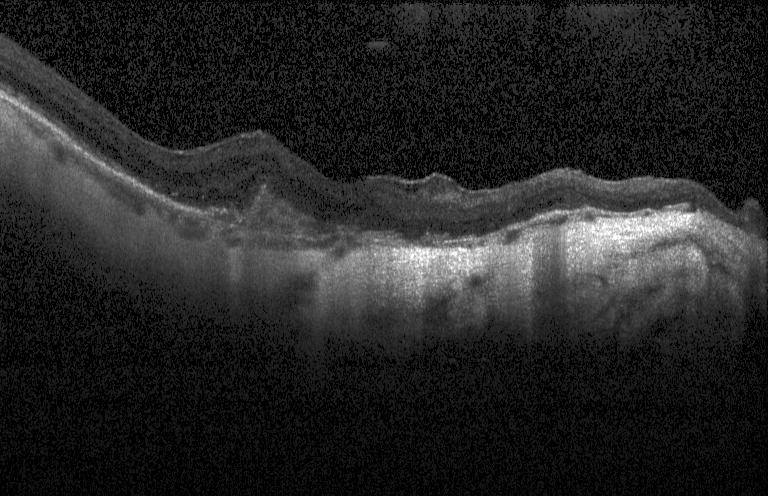

OCT B-scan showing a choroidal neovascular membrane.